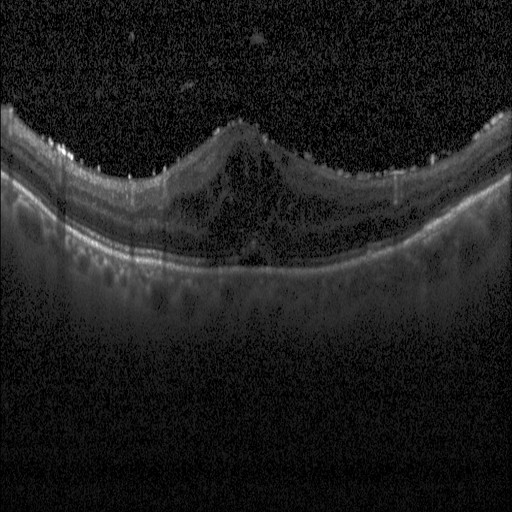
Impression: DME.